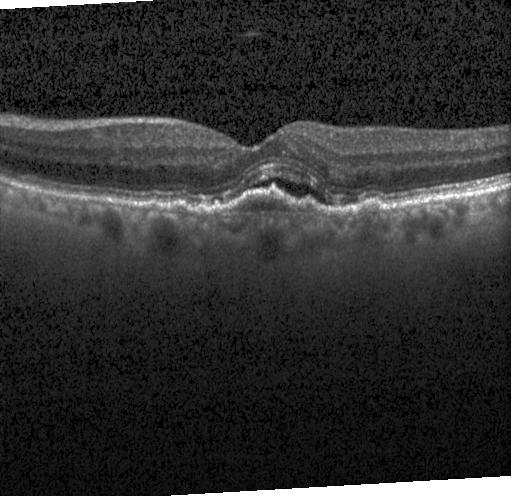
Retinal OCT cross-section; spectral-domain optical coherence tomography; centered on the fovea; Heidelberg Spectralis OCT system — The scan shows a choroidal neovascular membrane.